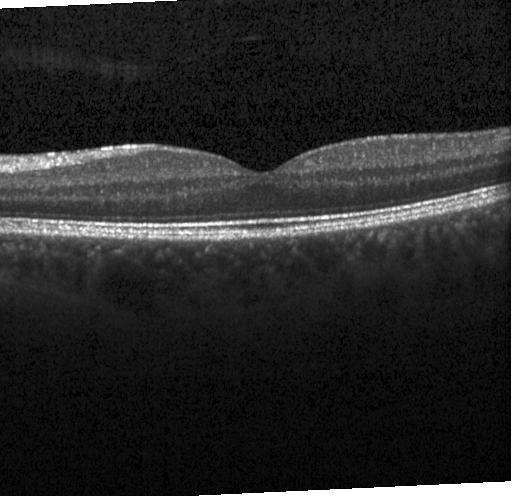

OCT scan showing no evidence of choroidal neovascularization, diabetic macular edema, or drusen.